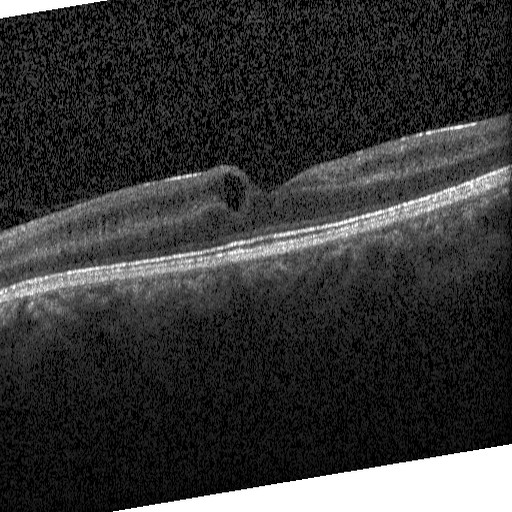

OCT line scan. Fovea-centered. SD-OCT. DME.